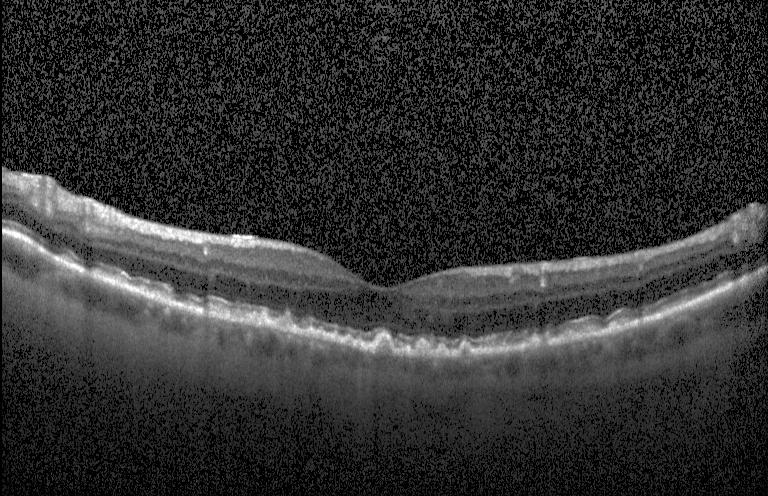

OCT B-scan, Heidelberg Spectralis.
Multiple drusen.